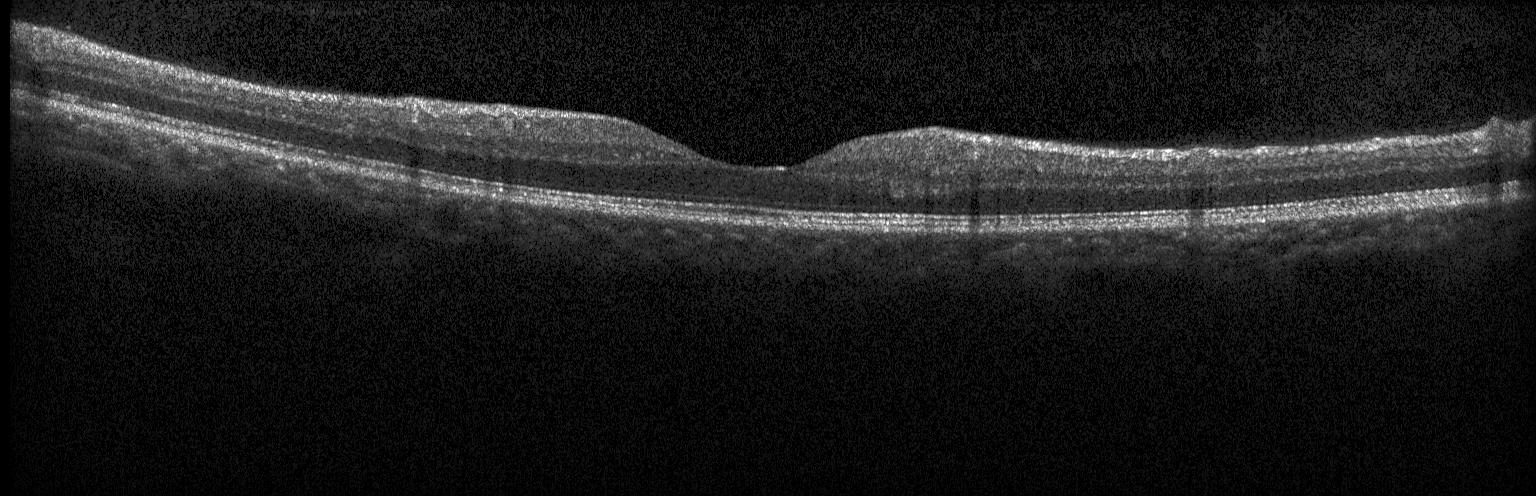 Centered on the fovea. Heidelberg Spectralis OCT system. SD-OCT. Retinal OCT cross-section.
The scan shows no evidence of CNV, DME, or drusen.